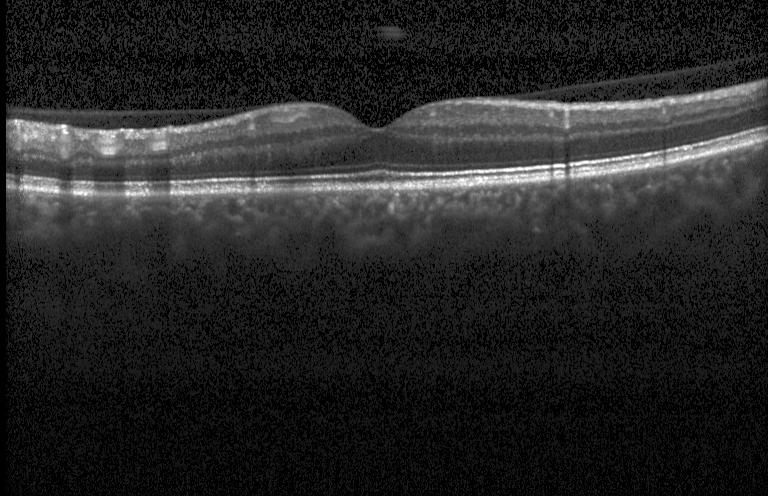

Impression: no evidence of choroidal neovascularization, diabetic macular edema, or drusen.